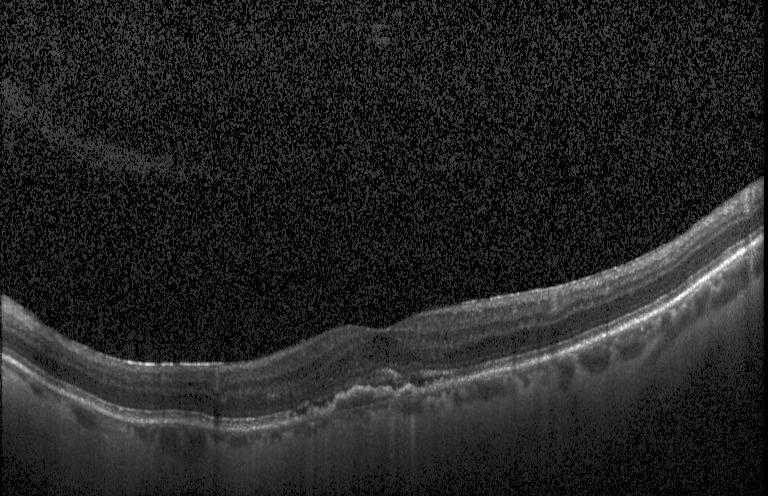

Optical coherence tomography scan · instrument: Heidelberg Spectralis
The scan shows a choroidal neovascular membrane.